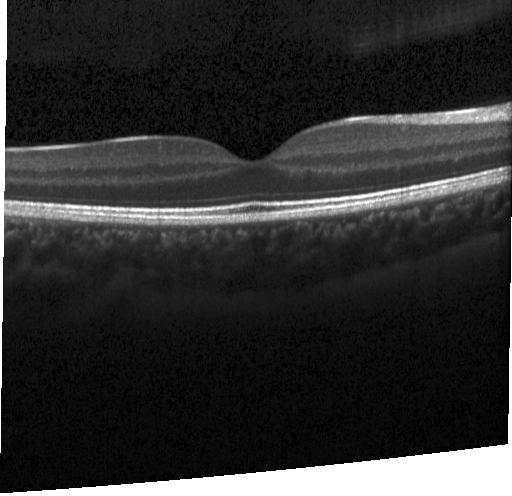 Retinal OCT cross-section showing neither choroidal neovascularization, diabetic macular edema, nor drusen.